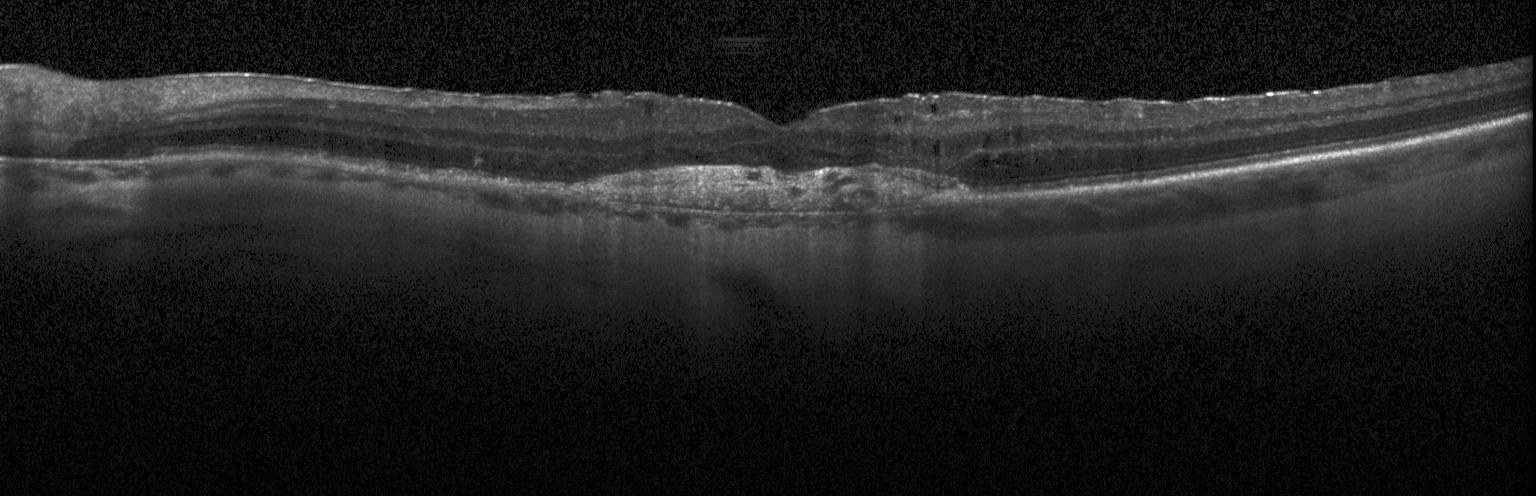
Retinal OCT cross-section · SD-OCT · Heidelberg Spectralis OCT system — Dx: a choroidal neovascular membrane.